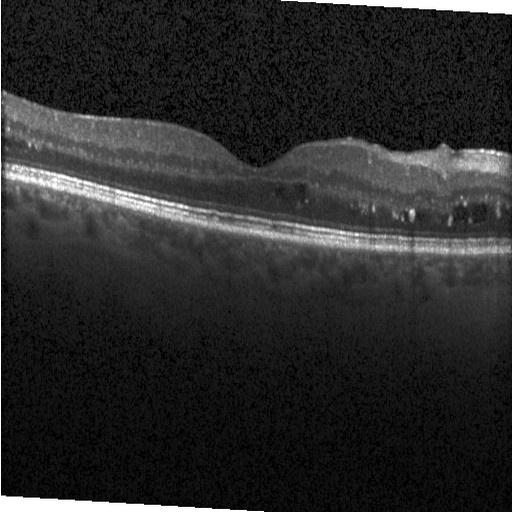

SD-OCT; Heidelberg Spectralis; optical coherence tomography scan.
The scan shows diabetic macular edema.